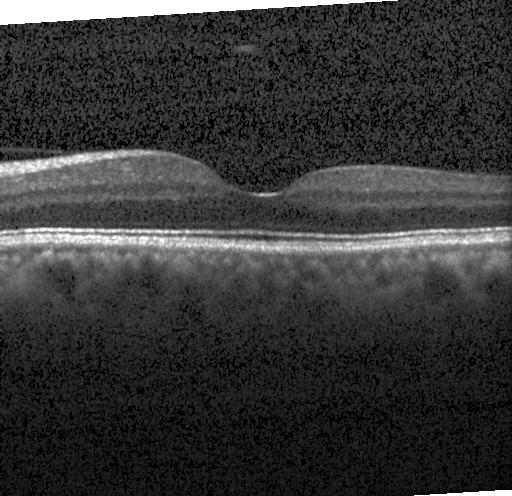 OCT B-scan showing no evidence of choroidal neovascularization, diabetic macular edema, or drusen.